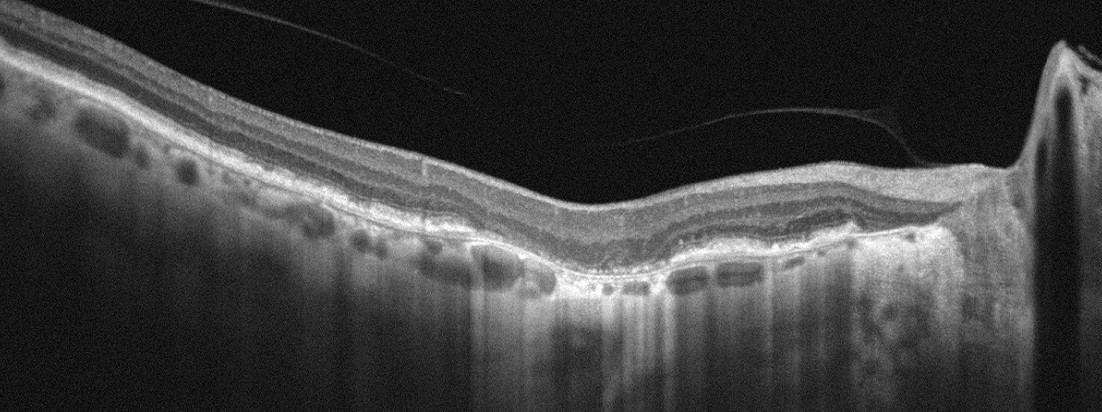 Spectral-domain OCT B-scan: age-related macular degeneration (AMD).